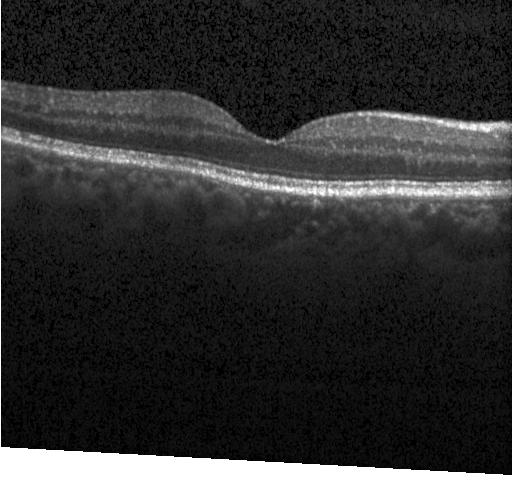
Diagnosis: neither choroidal neovascularization, diabetic macular edema, nor drusen.